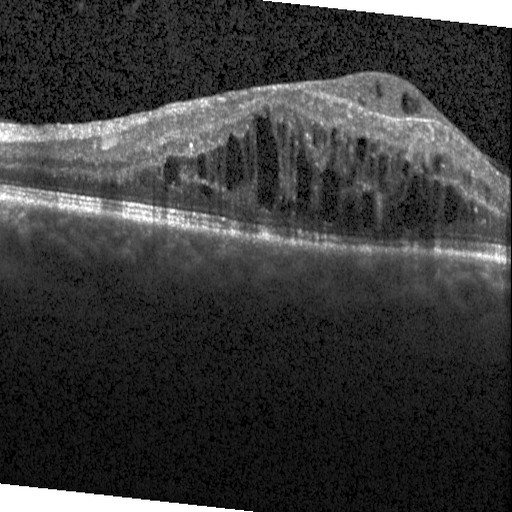
Macular scan, OCT B-scan, acquired on a Heidelberg Spectralis, SD-OCT.
Dx: DME.